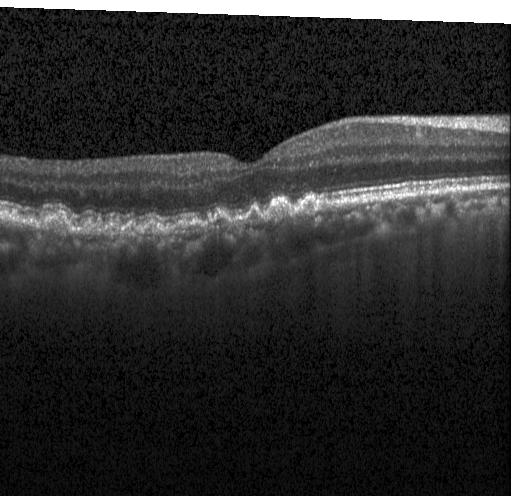 Optical coherence tomography B-scan. Diagnosis: drusen.